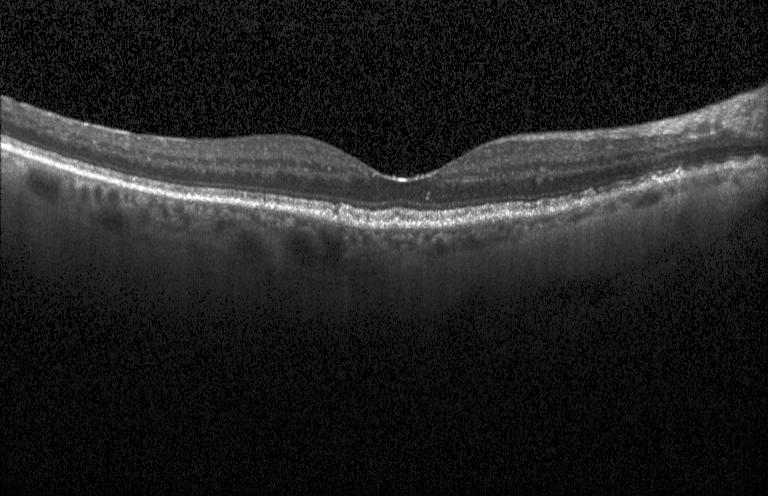 OCT finding: sub-RPE drusenoid deposits.